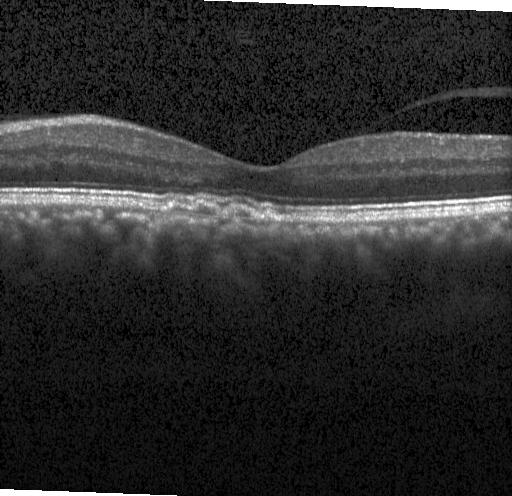
Through the macula · retinal OCT B-scan · spectral-domain optical coherence tomography. The scan shows drusen.